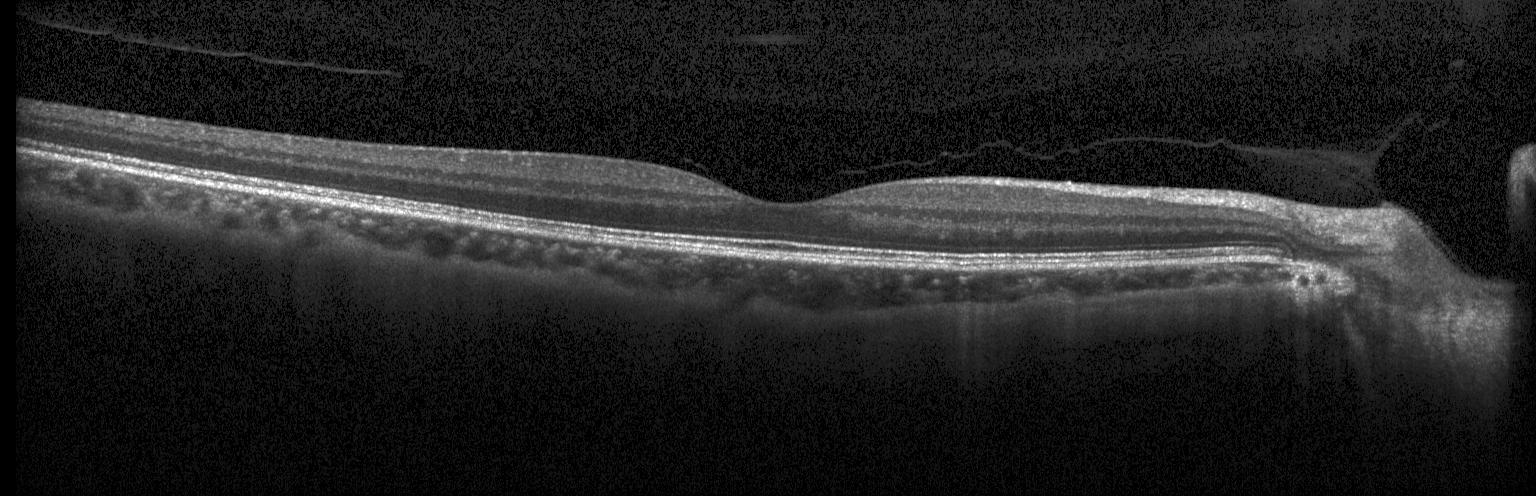
OCT B-scan
Impression: no CNV, no DME, and no drusen.